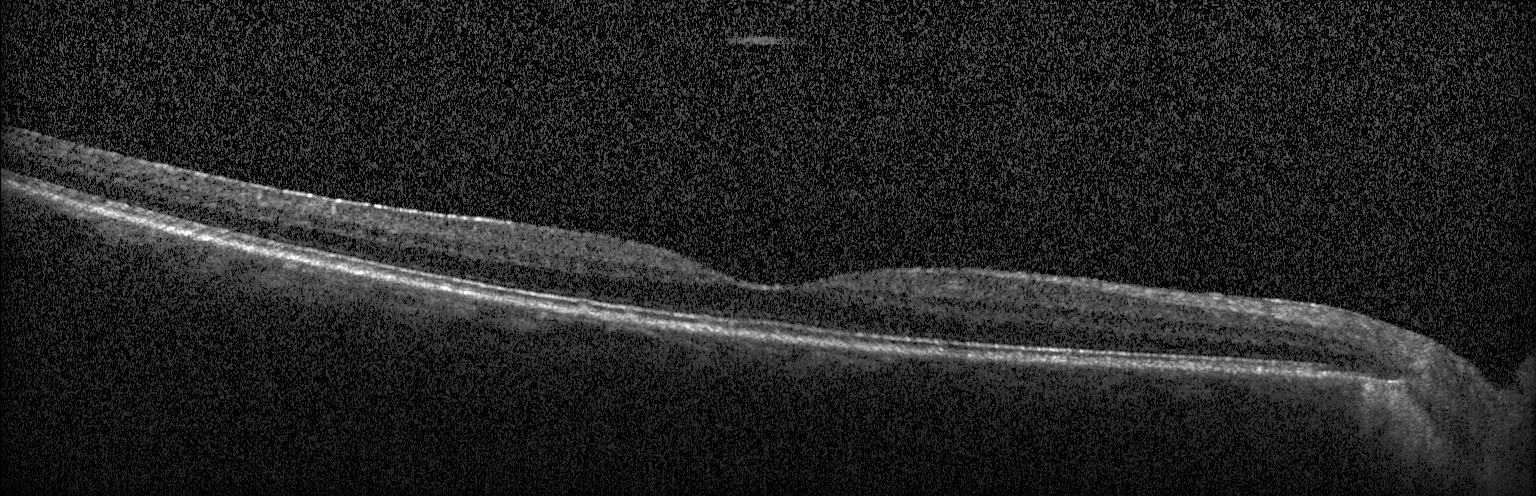 Impression: no evidence of choroidal neovascularization, diabetic macular edema, or drusen.